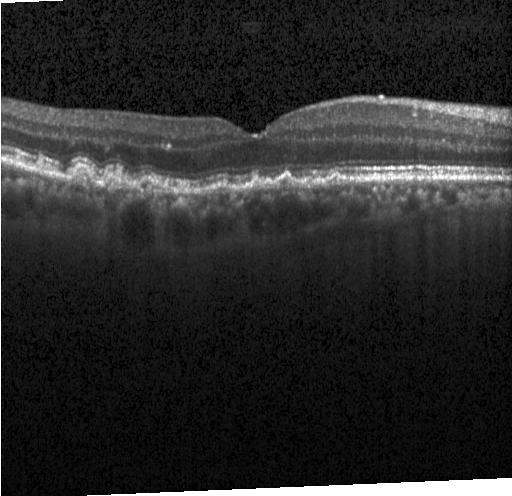

Retinal OCT B-scan. Horizontal scan through the fovea.
Dx: multiple drusen.